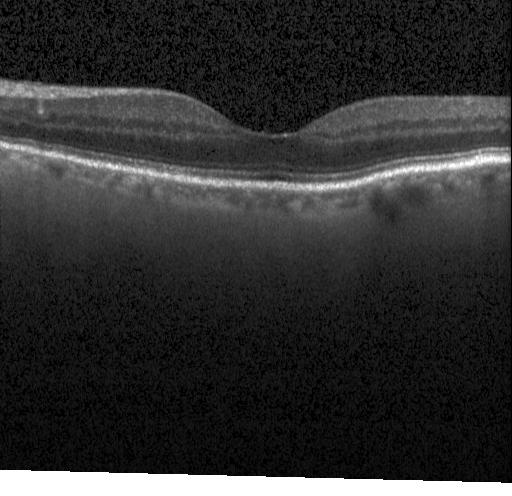 Centered on the fovea; spectral-domain OCT; Heidelberg Spectralis; retinal OCT B-scan.
Dx: no choroidal neovascularization, no diabetic macular edema, and no drusen.